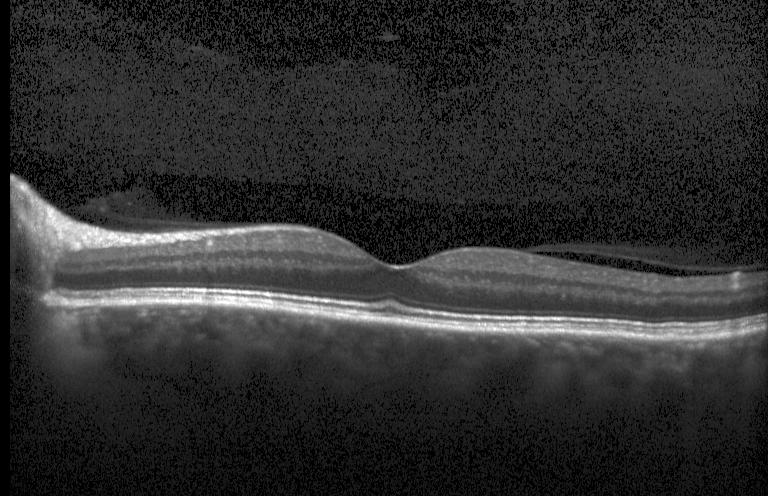
Spectral-domain OCT; fovea-centered; retinal OCT B-scan — This B-scan demonstrates no CNV, DME, or drusen.